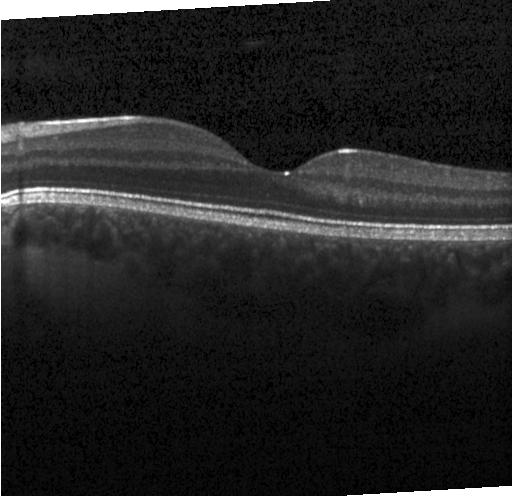
Acquired on a Heidelberg Spectralis, optical coherence tomography B-scan, horizontal scan through the fovea
Diagnosis: no evidence of CNV, DME, or drusen.